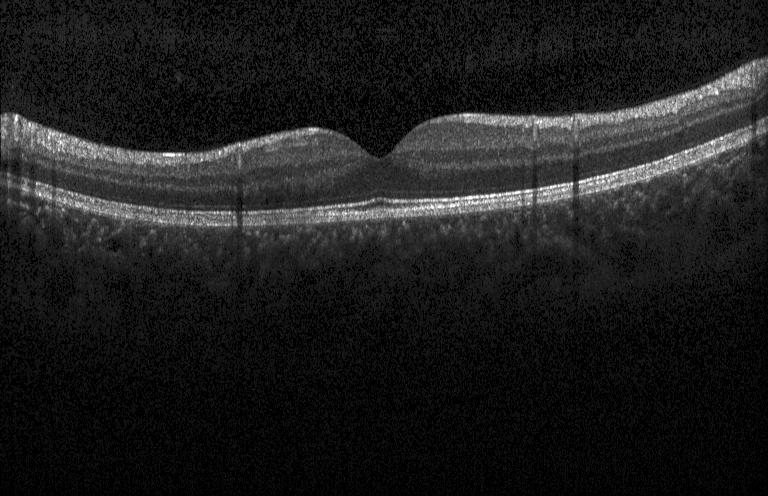
Spectral-domain OCT; Heidelberg Spectralis; centered on the fovea; OCT line scan. The scan shows no evidence of choroidal neovascularization, diabetic macular edema, or drusen.